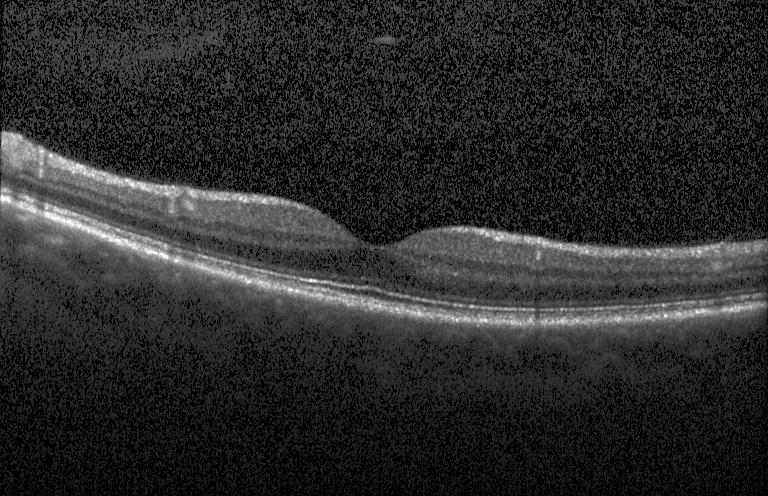 OCT B-scan.
Assessment: neither choroidal neovascularization, diabetic macular edema, nor drusen.